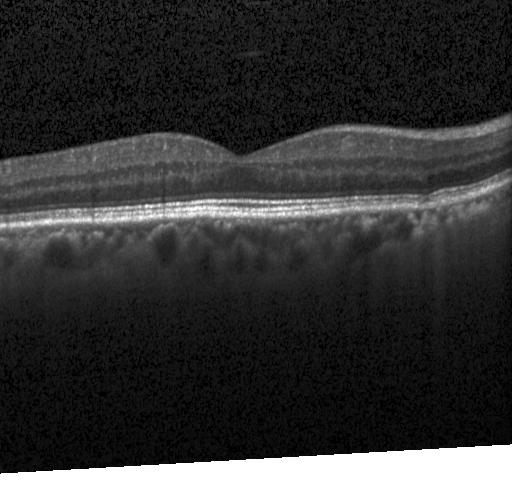 OCT B-scan · SD-OCT · acquired on a Heidelberg Spectralis · horizontal scan through the fovea. The scan shows no CNV, no DME, and no drusen.